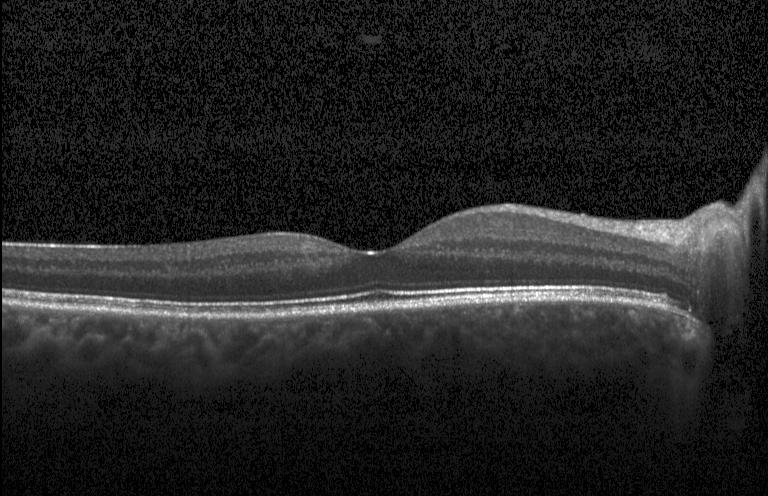
Through the macula, Heidelberg Spectralis, OCT B-scan
Assessment: neither CNV, DME, nor drusen.